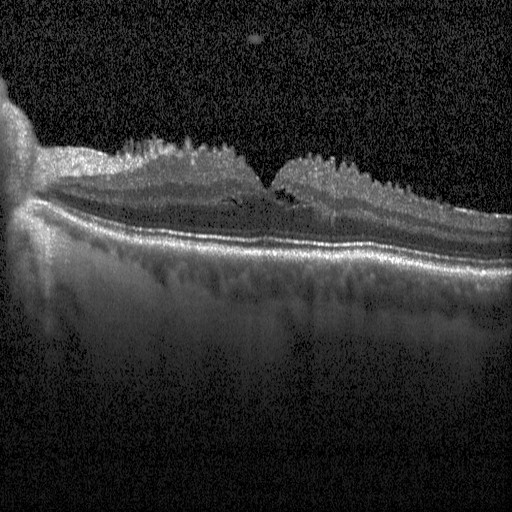
This B-scan demonstrates DME.